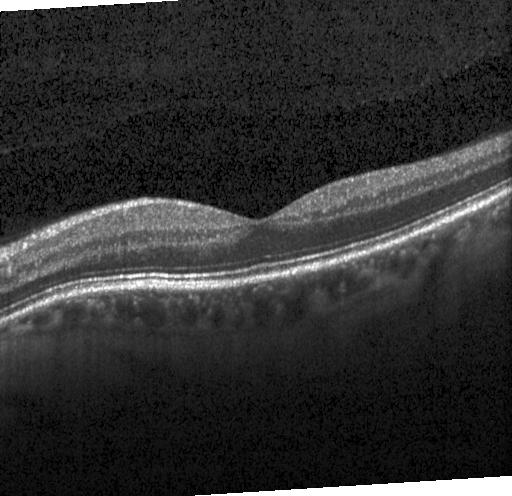 Impression: neither CNV, DME, nor drusen.